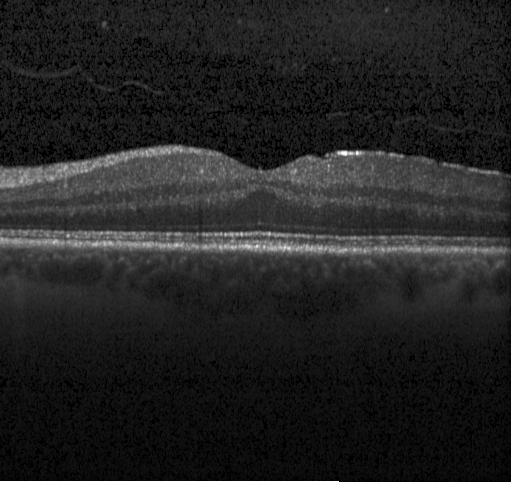
This B-scan demonstrates no choroidal neovascularization, no diabetic macular edema, and no drusen.